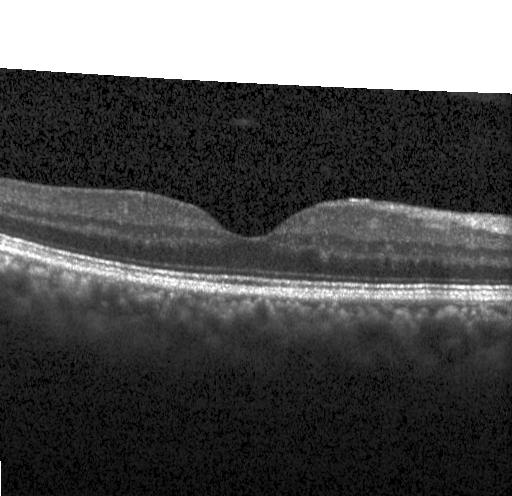
OCT line scan. Through the macula. Instrument: Heidelberg Spectralis. SD-OCT.
Impression: no choroidal neovascularization, diabetic macular edema, or drusen.